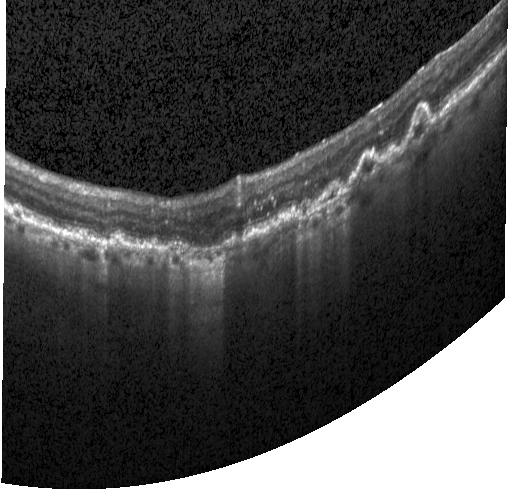 Horizontal scan through the fovea · instrument: Heidelberg Spectralis · optical coherence tomography scan
Finding: CNV.